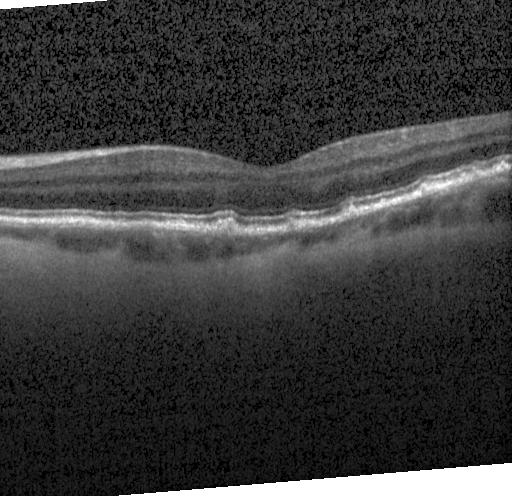
The scan shows multiple drusen.